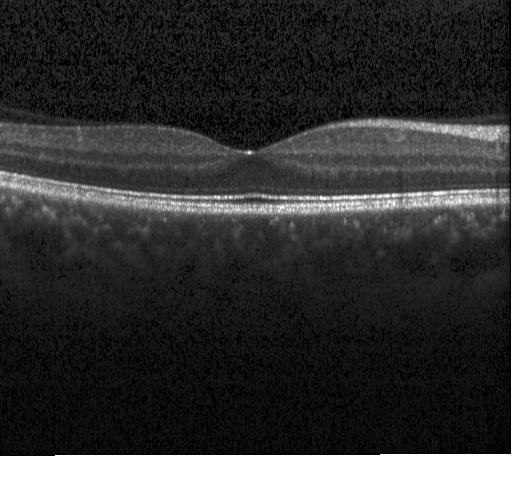
Spectral-domain OCT B-scan: neither choroidal neovascularization, diabetic macular edema, nor drusen.